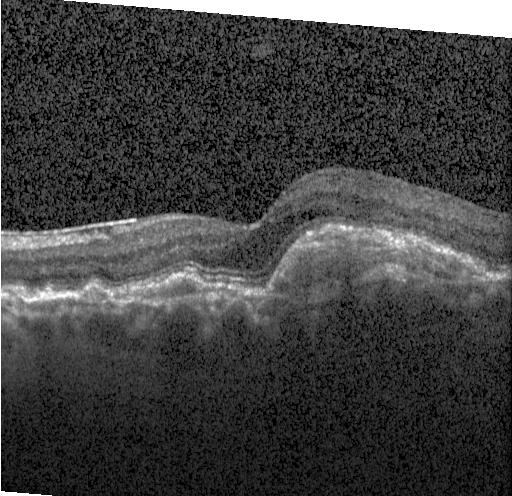 Dx: choroidal neovascularization.